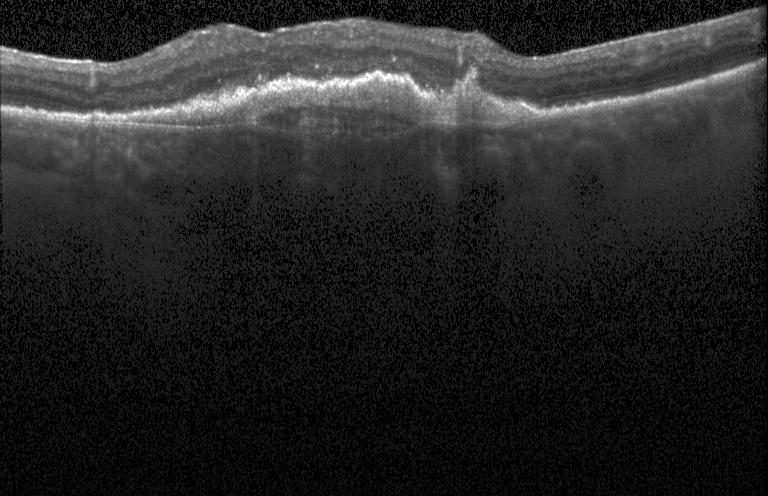

OCT scan showing a choroidal neovascular membrane.